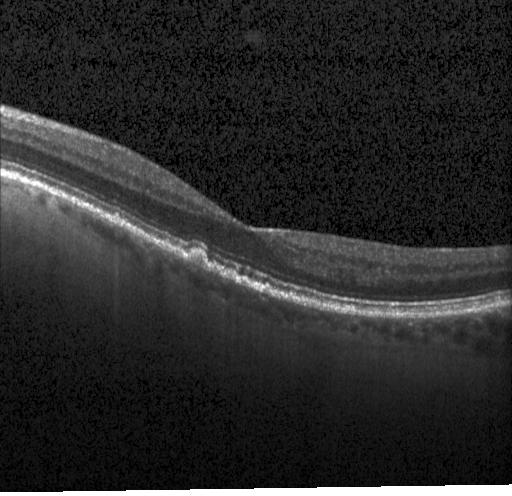

OCT line scan — Impression: multiple drusen.